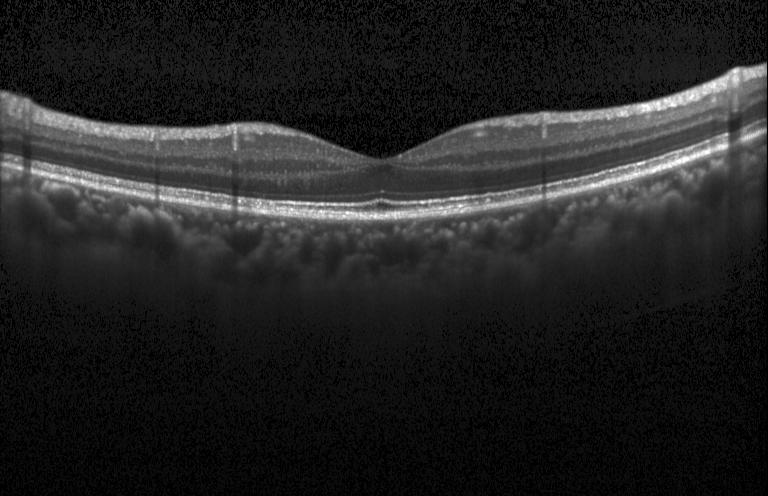

Impression: no evidence of CNV, DME, or drusen.